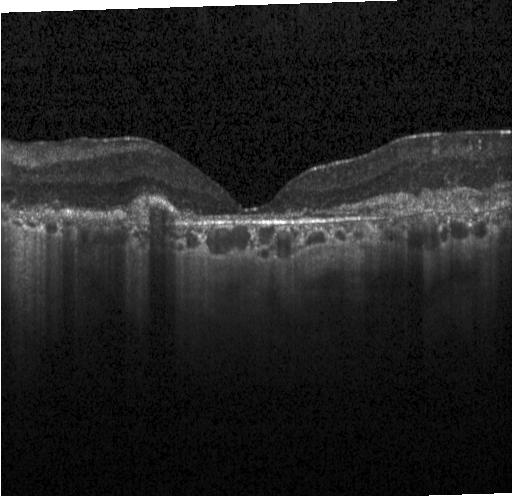
OCT finding: CNV.